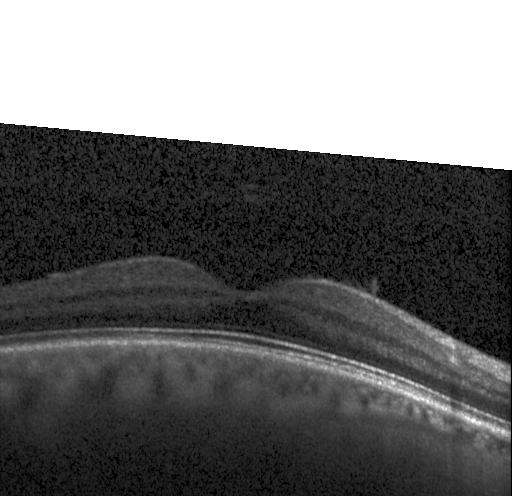

Optical coherence tomography scan, spectral-domain optical coherence tomography, Heidelberg Spectralis OCT system. Diagnosis: neither choroidal neovascularization, diabetic macular edema, nor drusen.